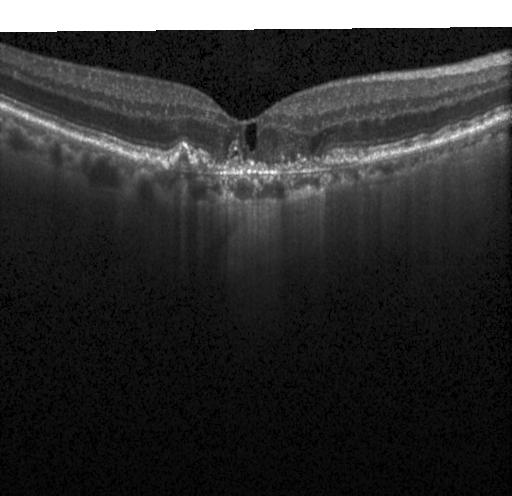

OCT B-scan. Macular OCT: a choroidal neovascular membrane.